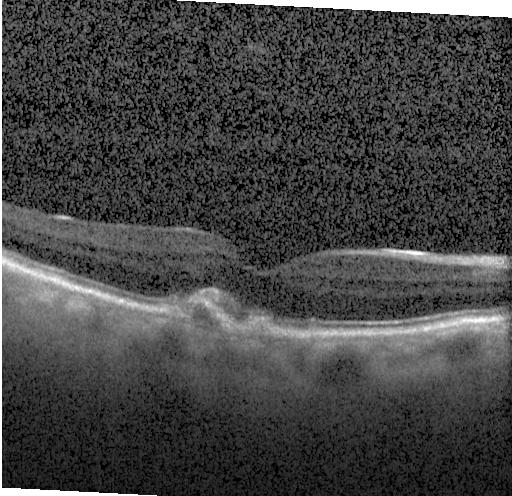
Retinal OCT cross-section · Heidelberg Spectralis OCT system
Finding: a choroidal neovascular membrane.